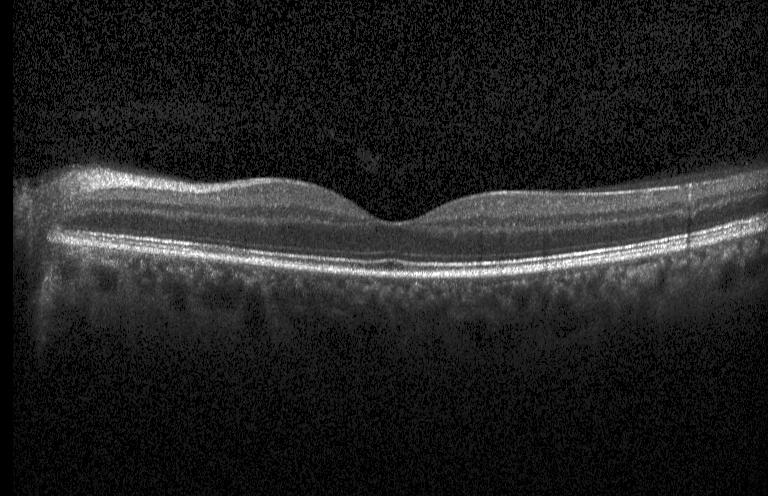
Centered on the fovea · Heidelberg Spectralis · optical coherence tomography B-scan · spectral-domain OCT.
Impression: no choroidal neovascularization, no diabetic macular edema, and no drusen.